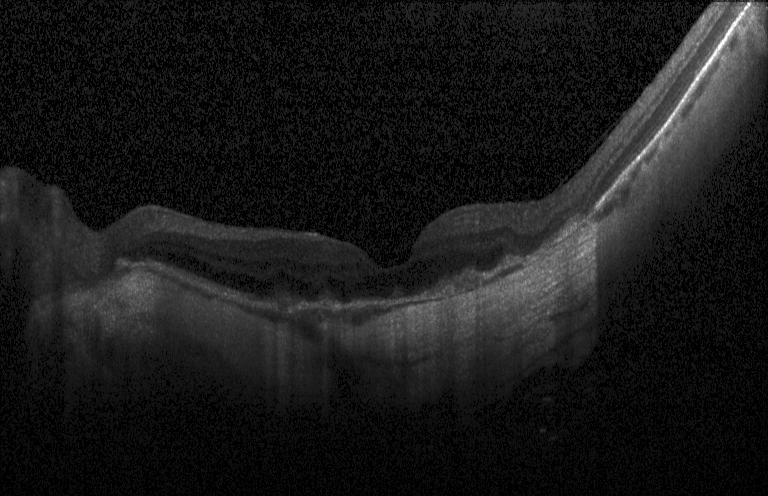

Acquired on a Heidelberg Spectralis; horizontal scan through the fovea; retinal OCT cross-section — Impression: a choroidal neovascular membrane.